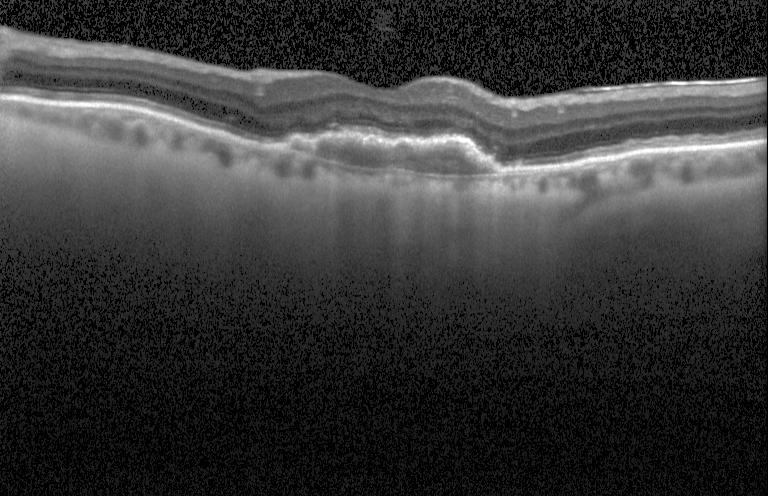

Optical coherence tomography scan — The scan shows choroidal neovascularization (CNV).